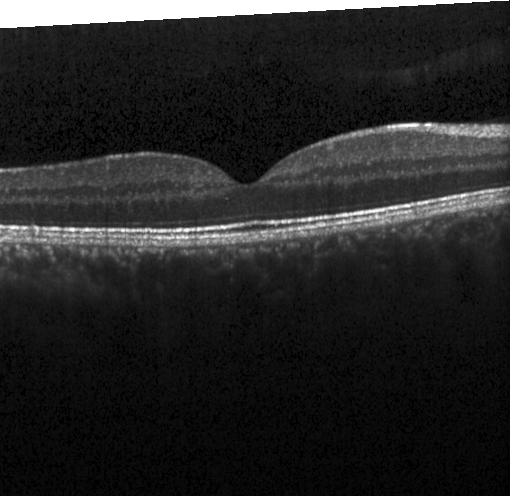

Finding: no evidence of choroidal neovascularization, diabetic macular edema, or drusen.